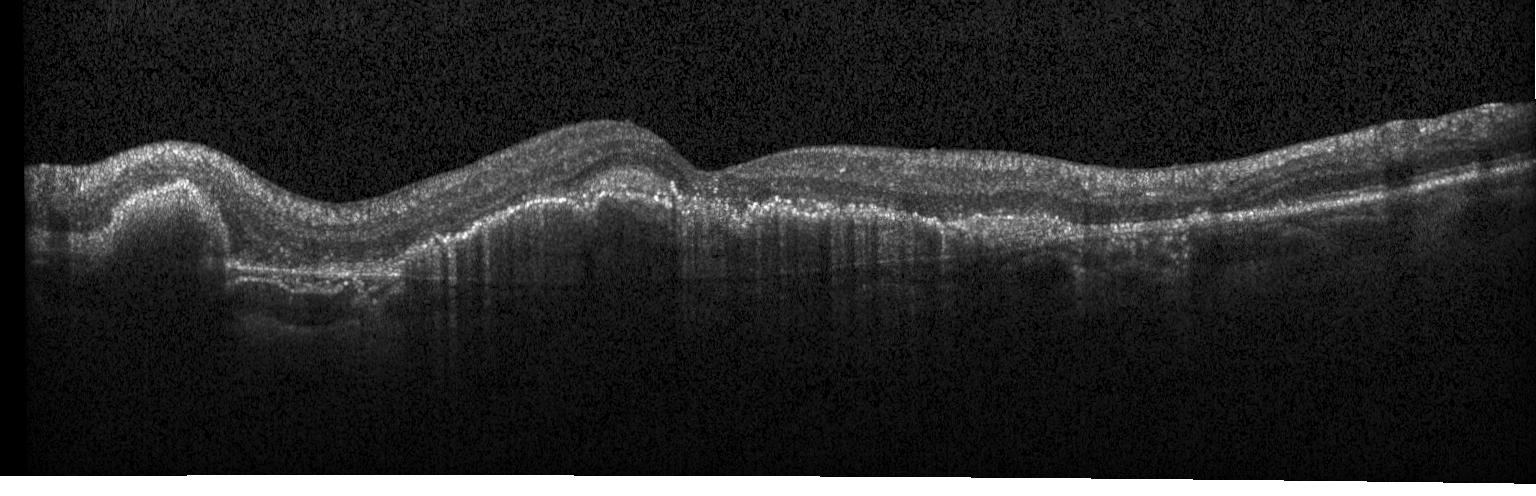
OCT scan showing a choroidal neovascular membrane.